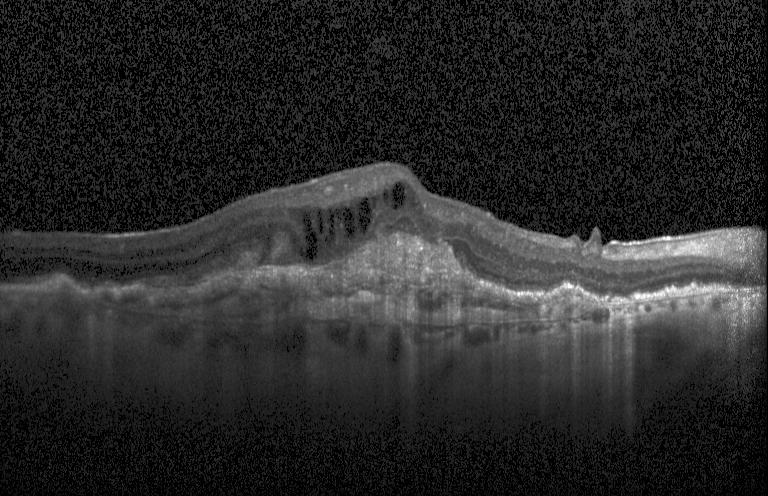
Fovea-centered, SD-OCT, optical coherence tomography scan. Macular OCT: a choroidal neovascular membrane.